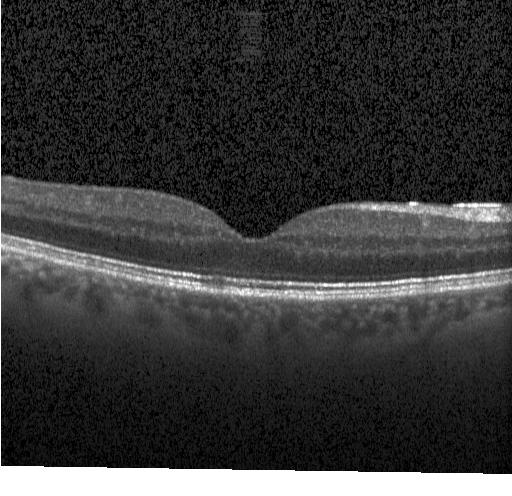 SD-OCT; OCT B-scan — Finding: neither choroidal neovascularization, diabetic macular edema, nor drusen.